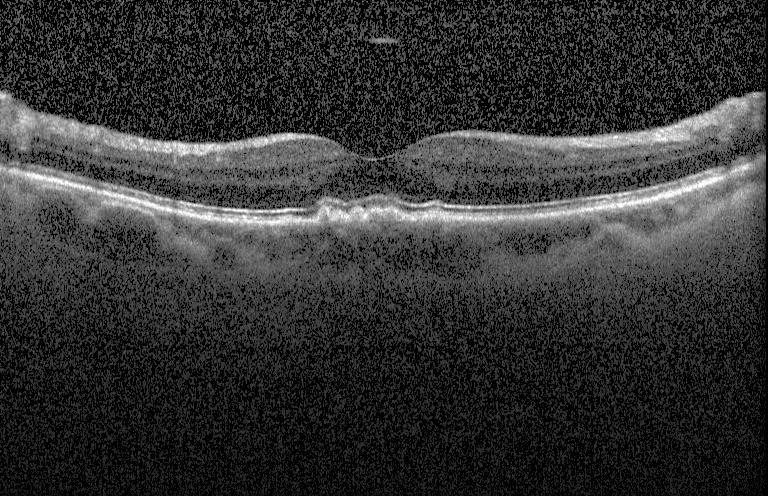
Optical coherence tomography B-scan · SD-OCT · instrument: Heidelberg Spectralis · fovea-centered — Finding: multiple drusen.